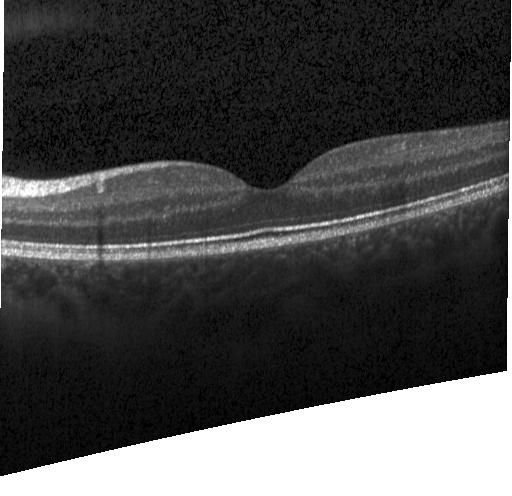
OCT B-scan showing no choroidal neovascularization, diabetic macular edema, or drusen.